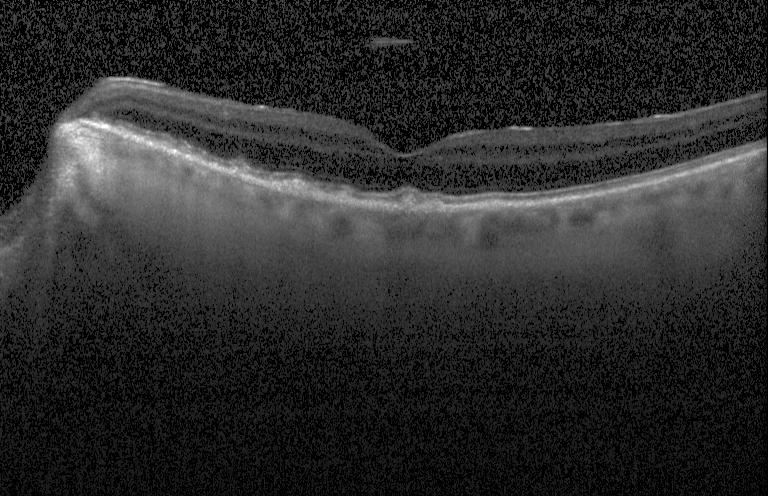 Horizontal scan through the fovea, retinal OCT B-scan — Impression: sub-RPE drusenoid deposits.